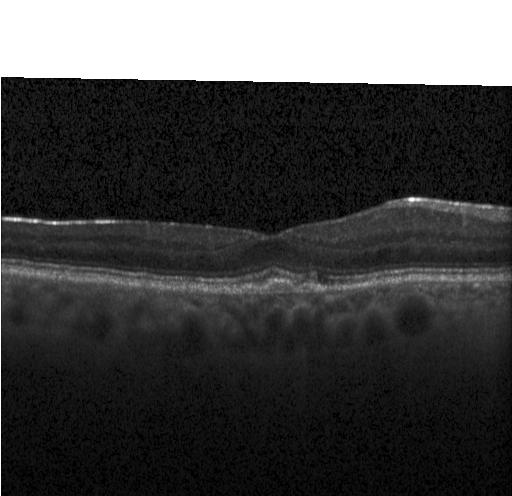 Optical coherence tomography B-scan
OCT finding: sub-RPE drusenoid deposits.